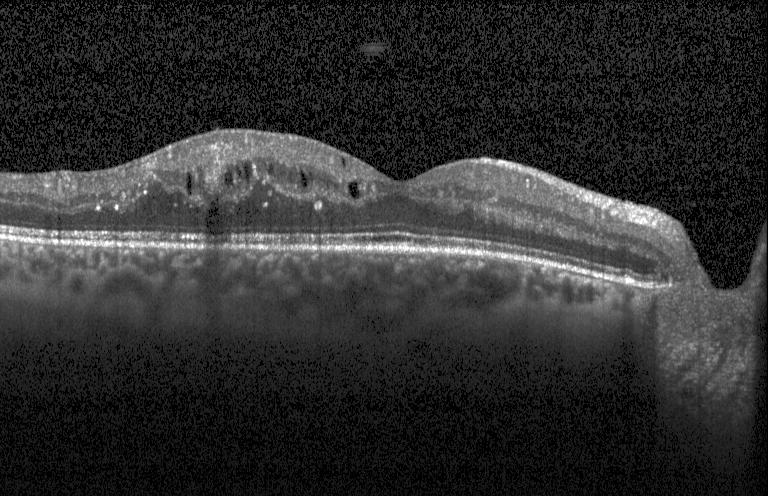
Macular scan; retinal OCT cross-section; instrument: Heidelberg Spectralis; spectral-domain OCT.
OCT finding: diabetic macular edema.